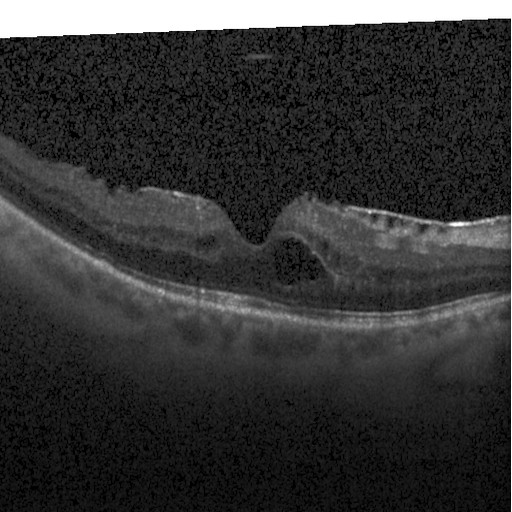

Spectral-domain optical coherence tomography. Retinal OCT B-scan. Acquired on a Heidelberg Spectralis.
OCT finding: diabetic macular edema.